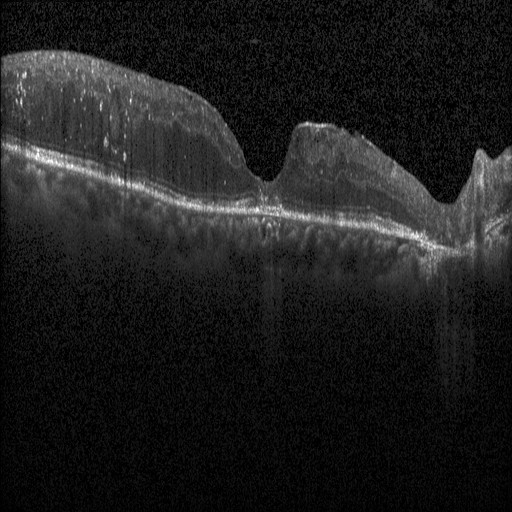

Macular OCT demonstrating diabetic macular edema.